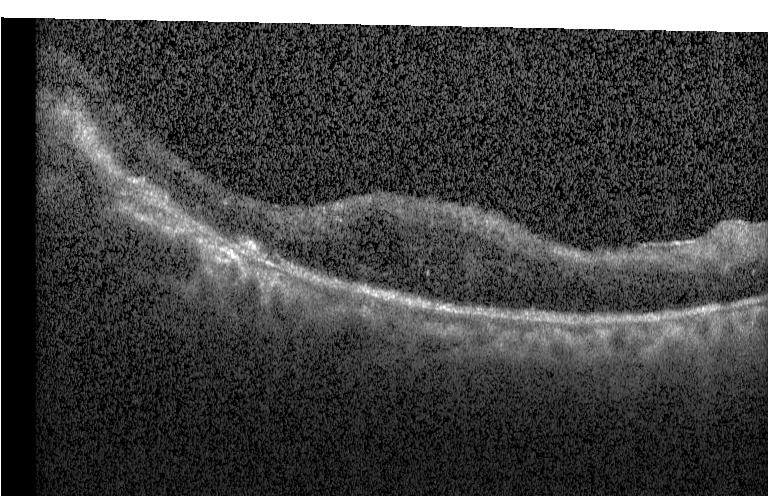
Impression: DME.